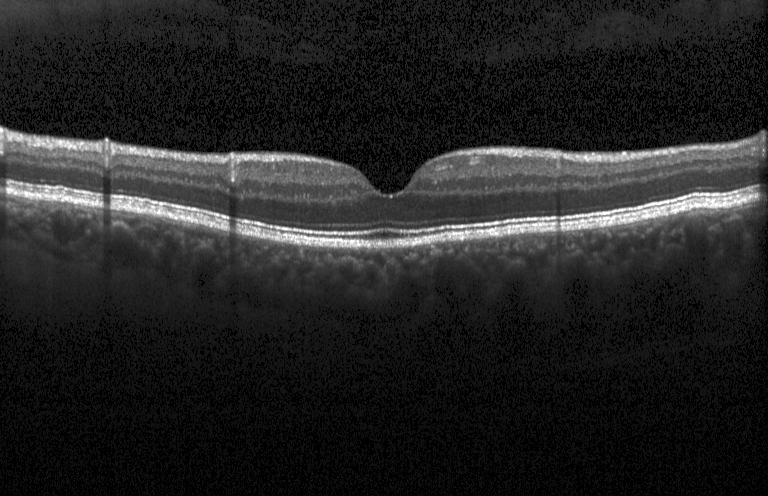
OCT B-scan showing no choroidal neovascularization, no diabetic macular edema, and no drusen.